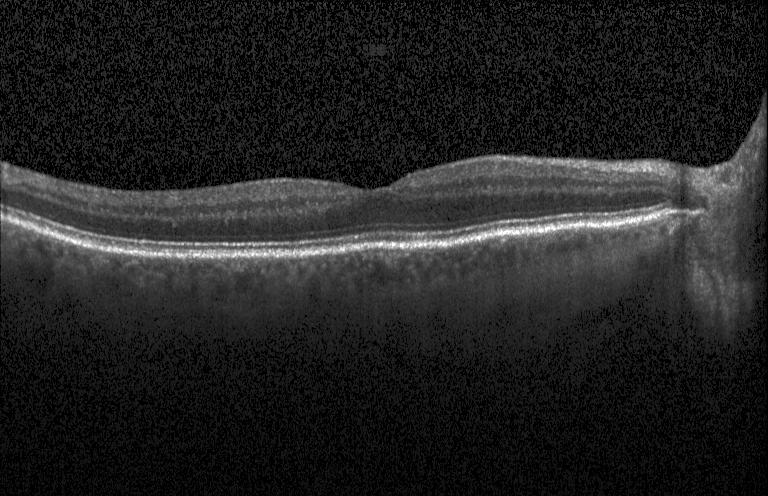 Heidelberg Spectralis OCT system; OCT line scan; spectral-domain OCT; horizontal scan through the fovea. This B-scan demonstrates neither CNV, DME, nor drusen.